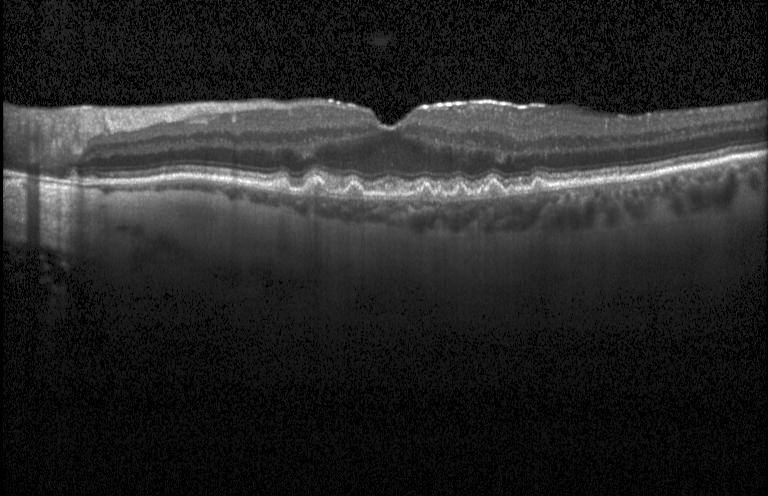 Impression: drusen.